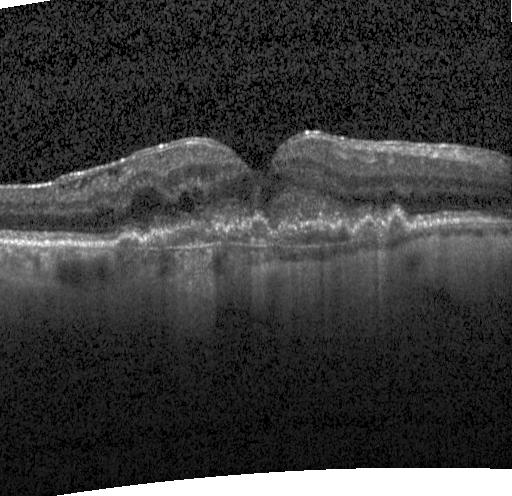 OCT B-scan · acquired on a Heidelberg Spectralis · centered on the fovea — Macular OCT: CNV.